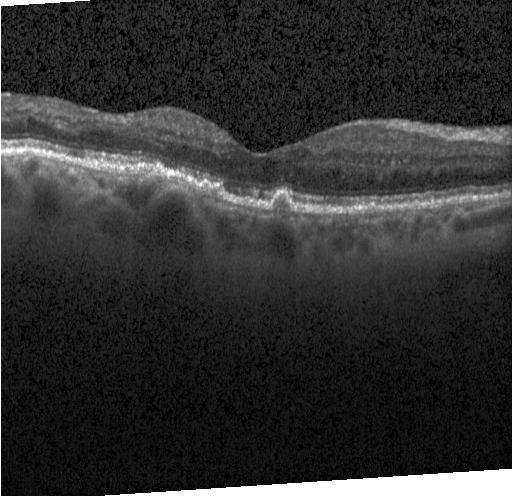
Sub-RPE drusenoid deposits.